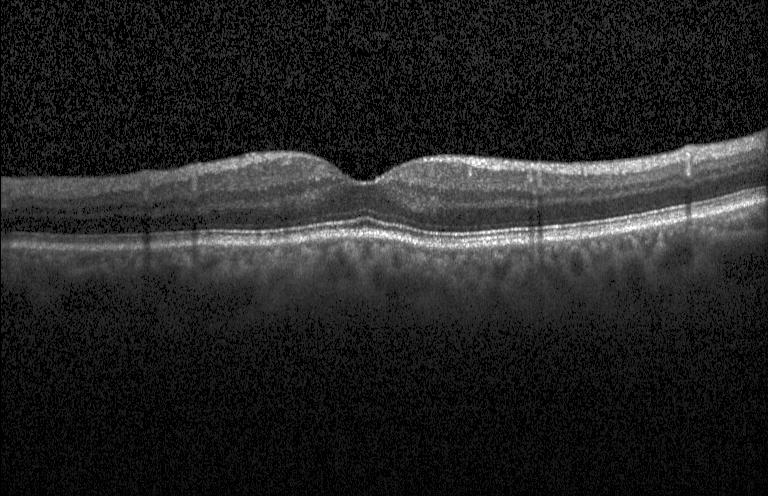

Optical coherence tomography scan; horizontal scan through the fovea. Macular OCT: neither CNV, DME, nor drusen.